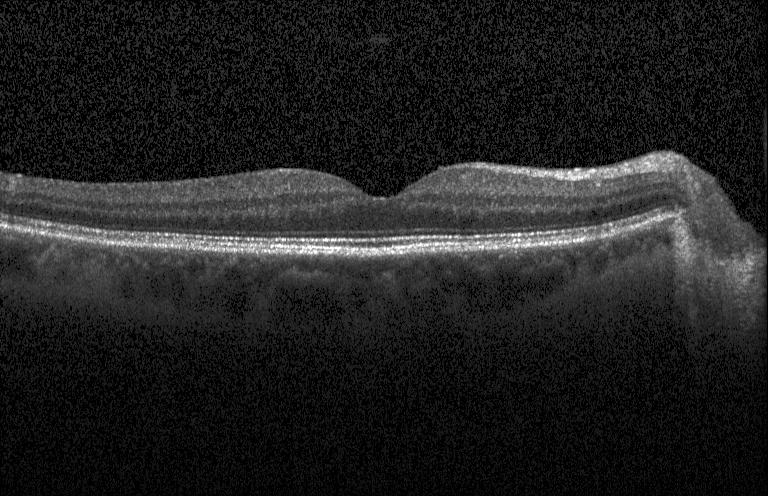 Impression: no choroidal neovascularization, no diabetic macular edema, and no drusen.